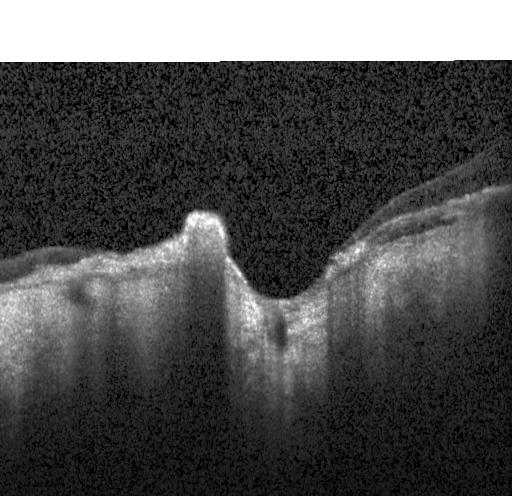

Heidelberg Spectralis. OCT B-scan. Fovea-centered.
Dx: CNV.